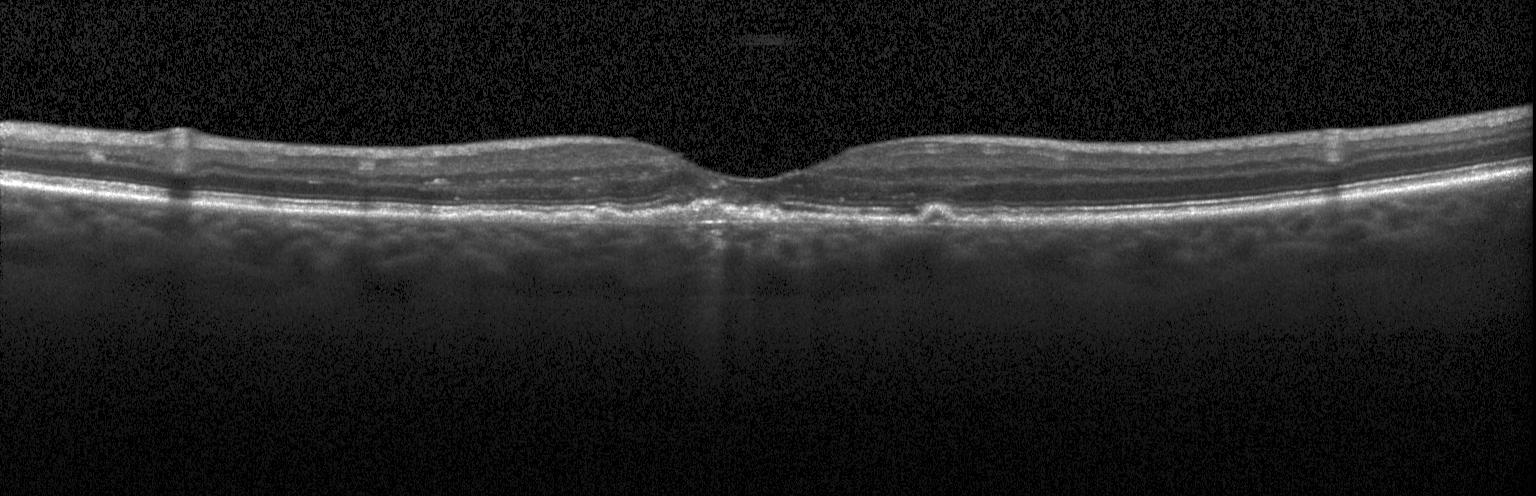

Finding: a choroidal neovascular membrane.